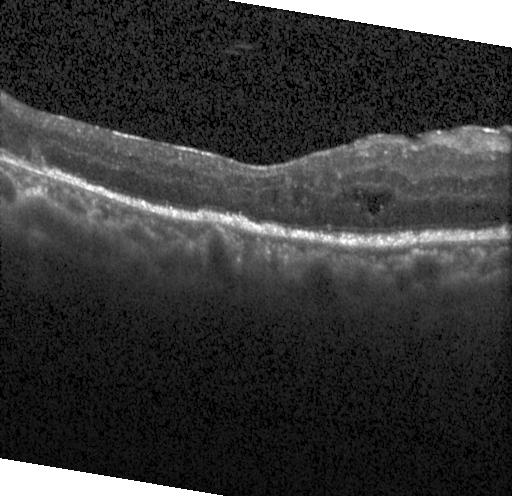

OCT B-scan. Diagnosis: diabetic macular edema (DME).